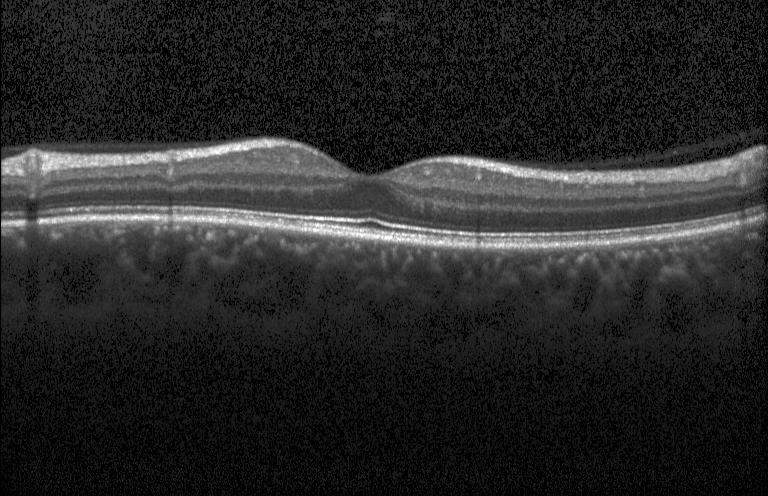

OCT line scan, horizontal scan through the fovea.
Finding: no evidence of choroidal neovascularization, diabetic macular edema, or drusen.